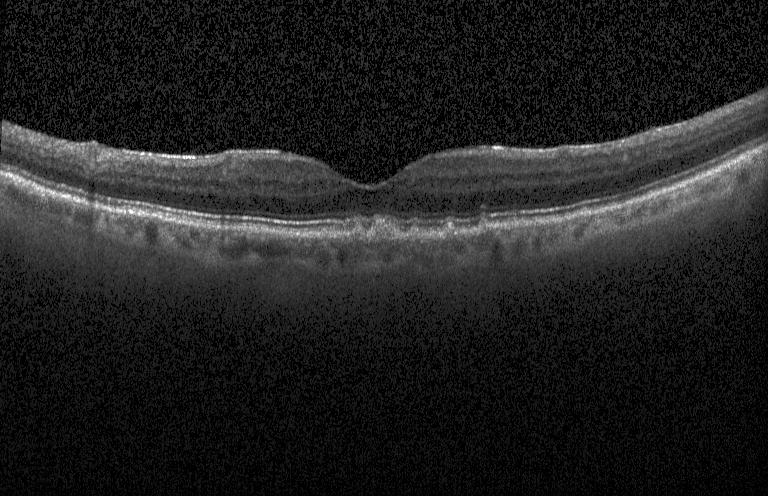

Assessment: drusen.